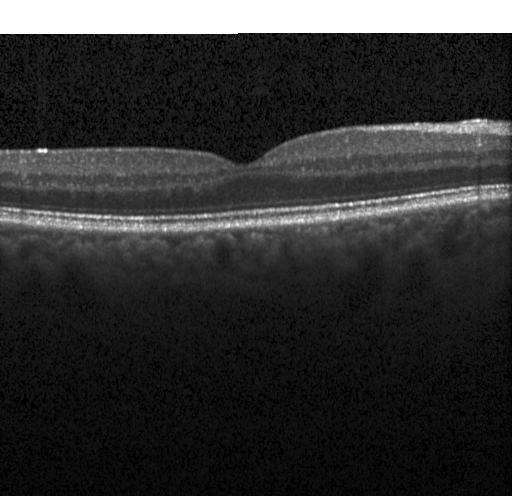
OCT finding: neither choroidal neovascularization, diabetic macular edema, nor drusen.